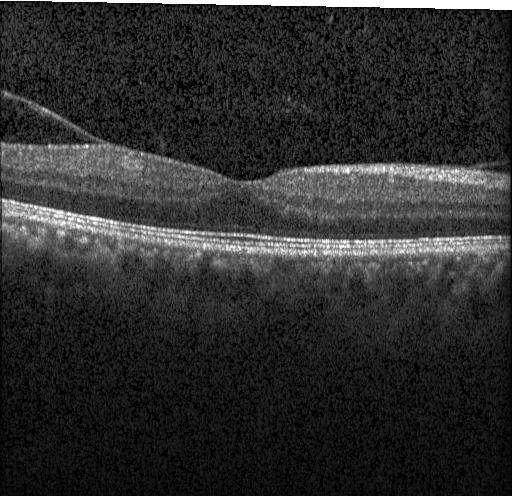
Optical coherence tomography scan.
Finding: no evidence of choroidal neovascularization, diabetic macular edema, or drusen.